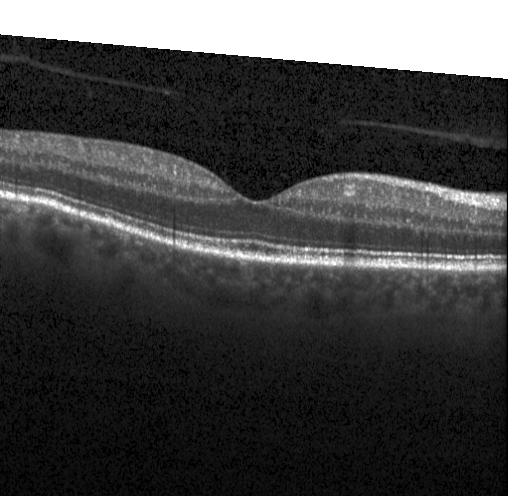

Spectral-domain OCT · retinal OCT cross-section · instrument: Heidelberg Spectralis.
Neither choroidal neovascularization, diabetic macular edema, nor drusen.